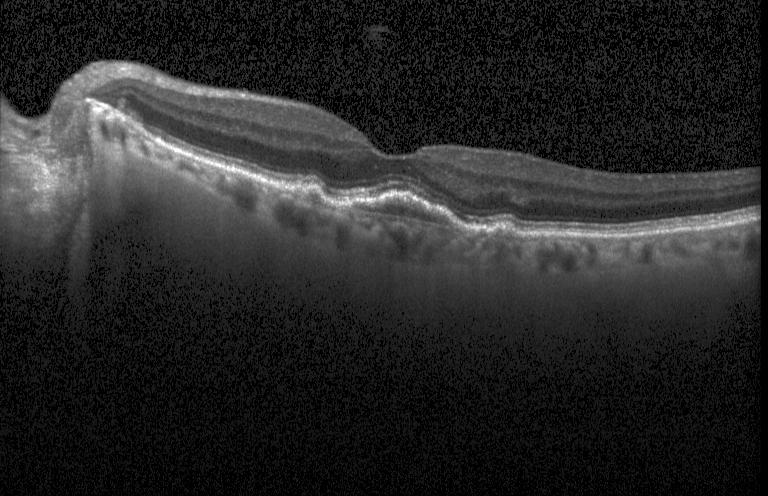
Through the macula, OCT B-scan, instrument: Heidelberg Spectralis, SD-OCT
Impression: a choroidal neovascular membrane.